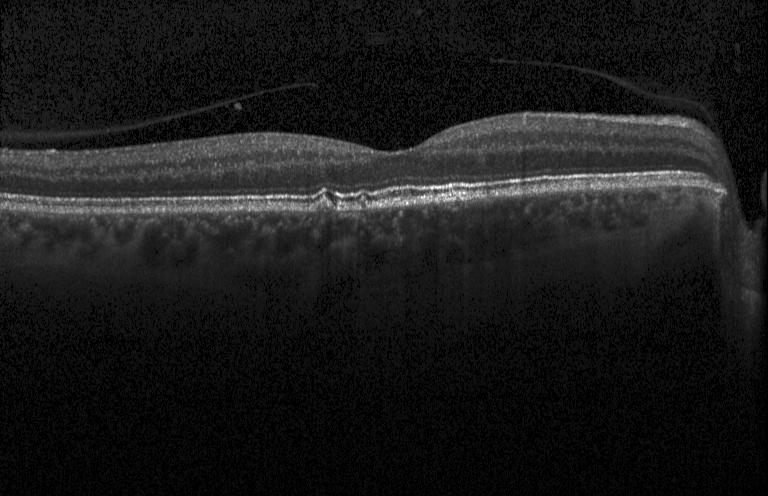
Centered on the fovea · optical coherence tomography scan.
Diagnosis: drusen.